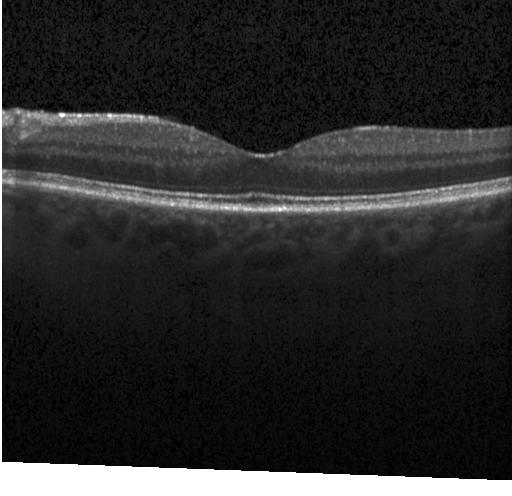
Retinal OCT cross-section. Through the macula. Finding: no evidence of choroidal neovascularization, diabetic macular edema, or drusen.